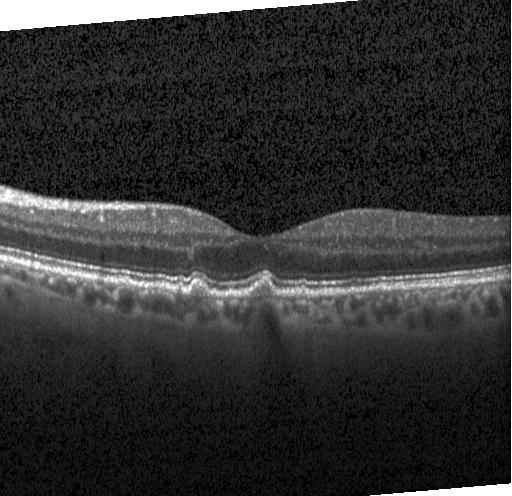 Retinal OCT cross-section — This B-scan demonstrates sub-RPE drusenoid deposits.